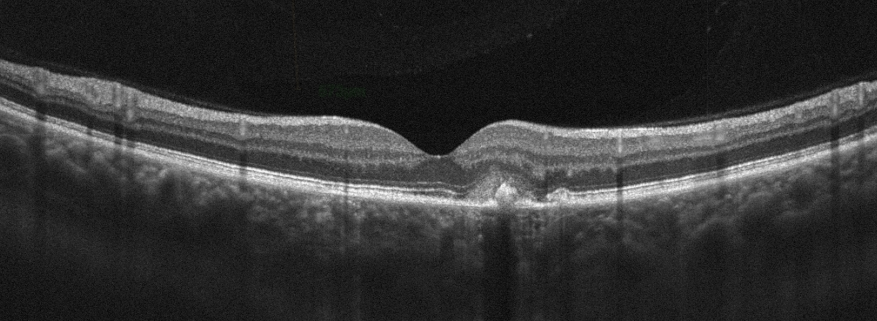

Acquired on an Optovue Avanti RTVue XR. Through the macula. OCT line scan. Diagnosis: age-related macular degeneration.